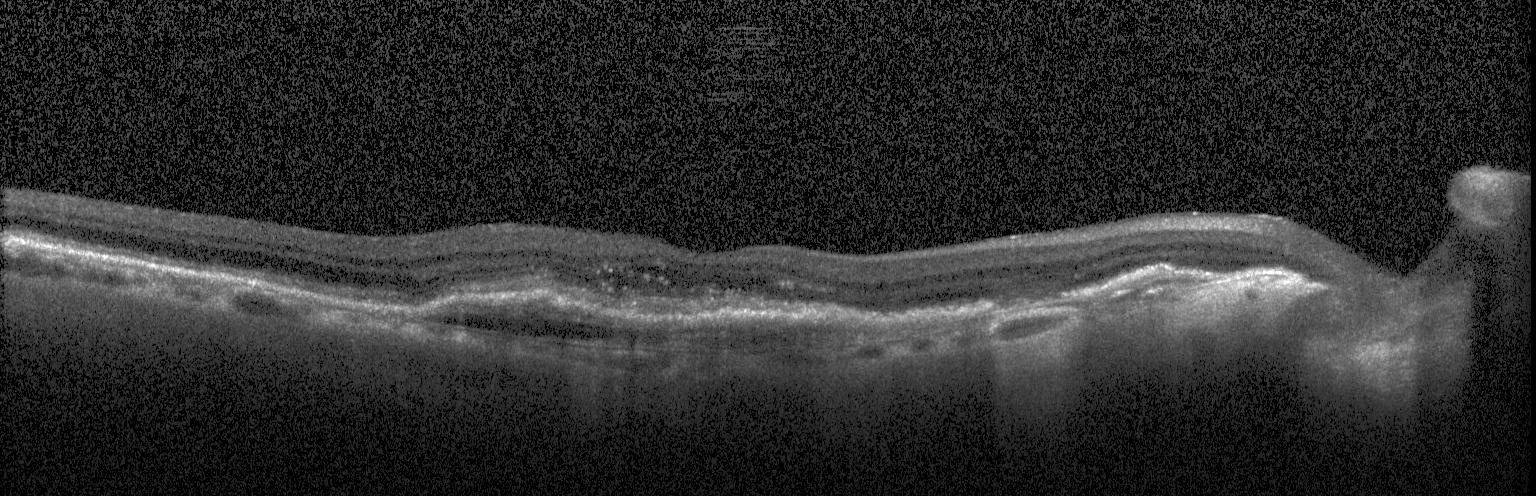 Macular OCT: choroidal neovascularization.